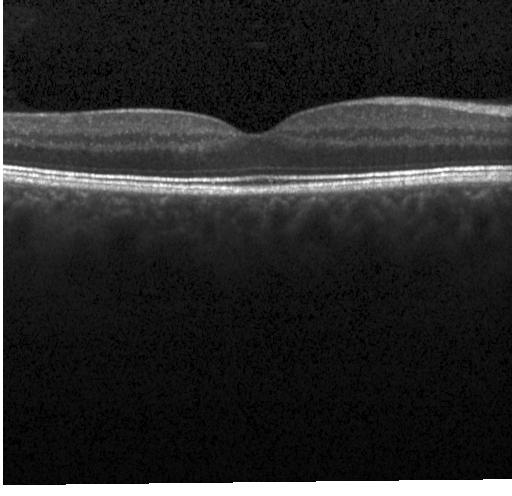 Impression: no choroidal neovascularization, no diabetic macular edema, and no drusen.